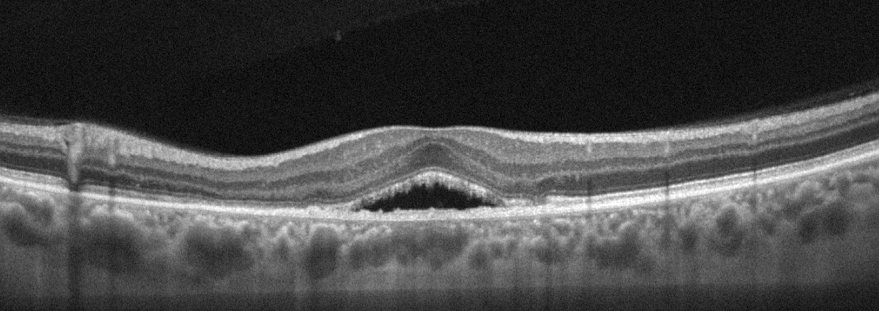
Retinal OCT cross-section showing age-related macular degeneration (AMD).